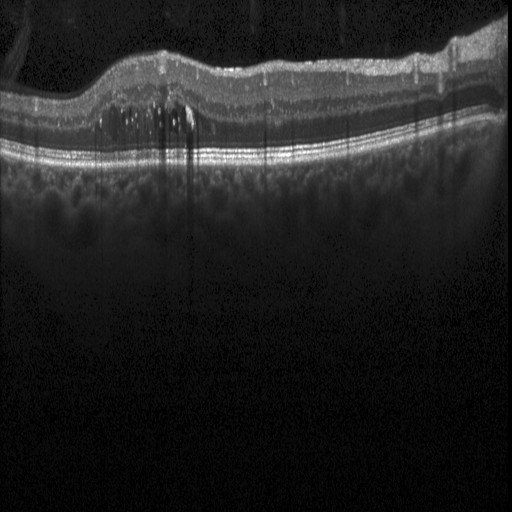
Diabetic macular edema.